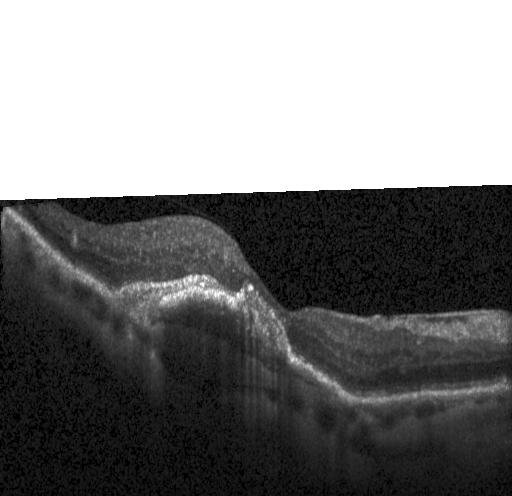
Spectral-domain OCT B-scan: choroidal neovascularization.